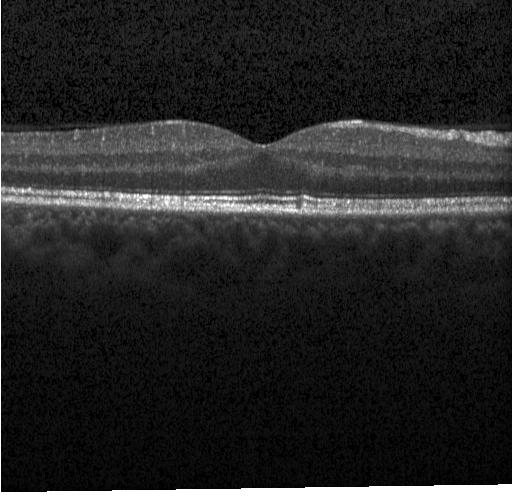 OCT B-scan showing neither CNV, DME, nor drusen.